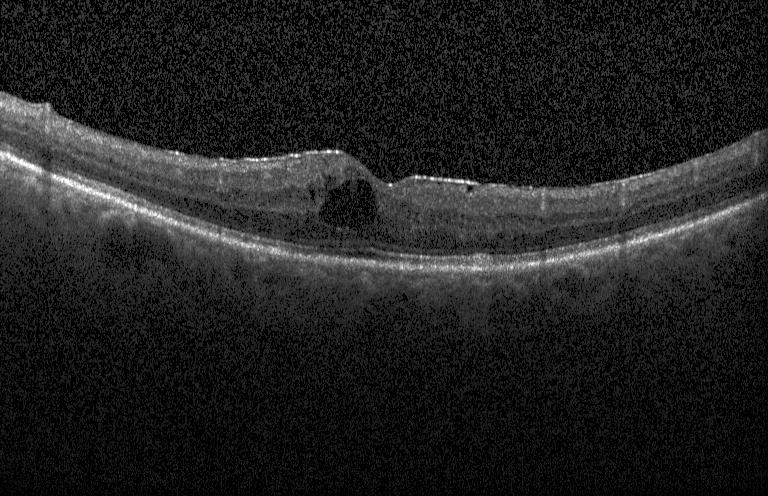 Optical coherence tomography B-scan, instrument: Heidelberg Spectralis, horizontal scan through the fovea, SD-OCT.
Diagnosis: DME.